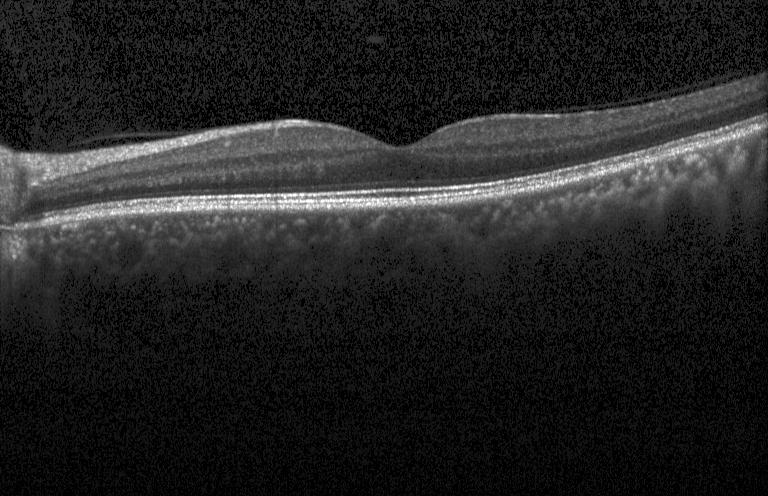 Assessment: neither choroidal neovascularization, diabetic macular edema, nor drusen.